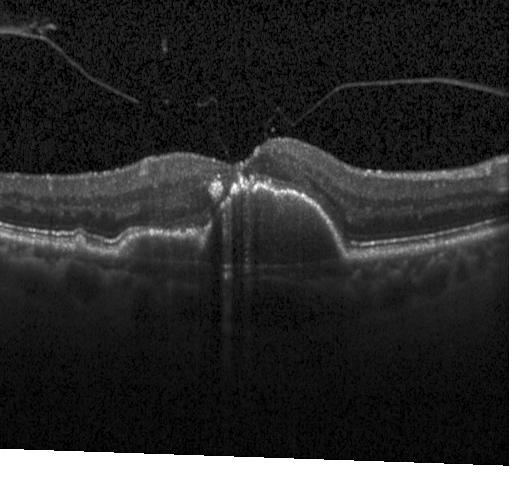 OCT B-scan. Impression: choroidal neovascularization.